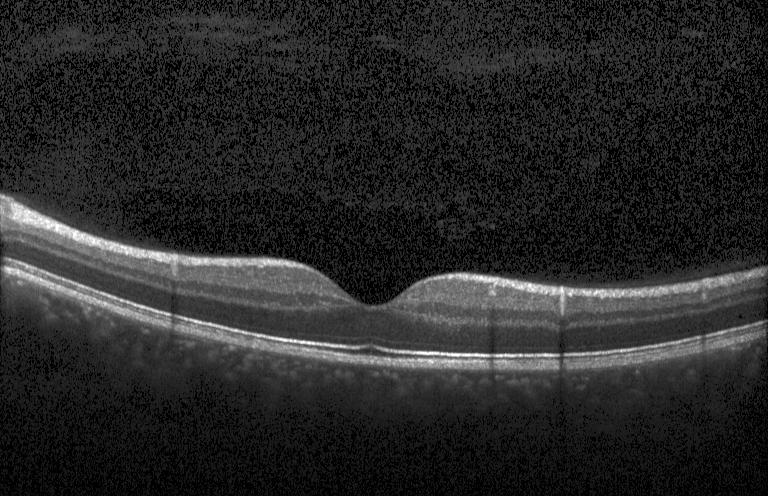 Optical coherence tomography scan. Finding: no evidence of CNV, DME, or drusen.